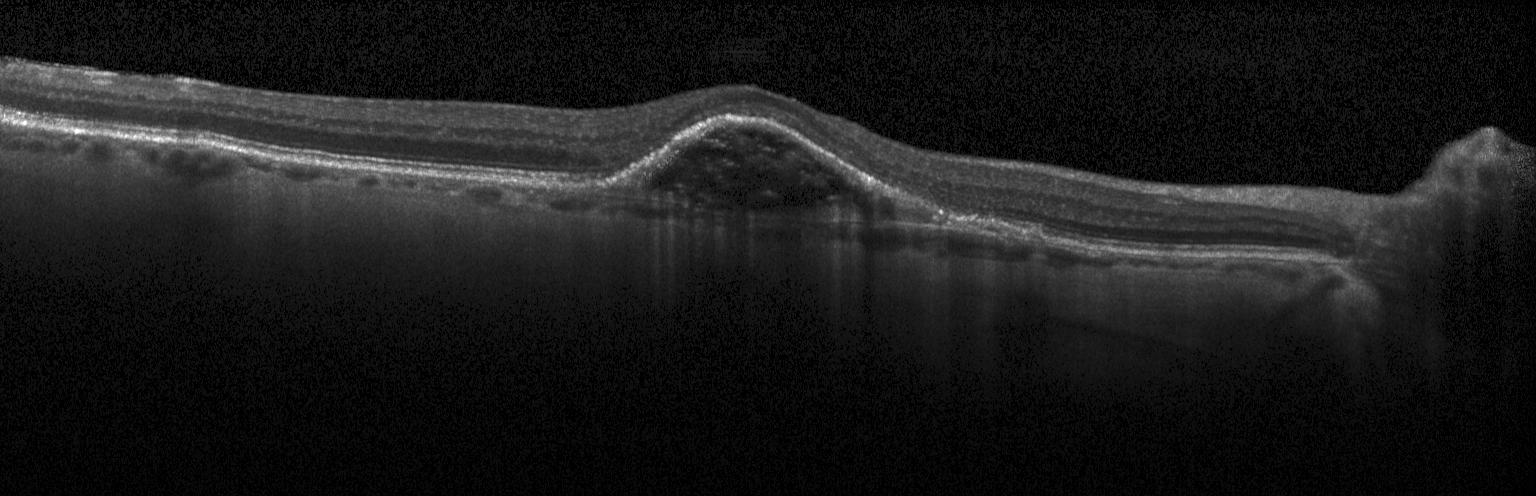

Horizontal scan through the fovea · optical coherence tomography scan · spectral-domain optical coherence tomography
Impression: a choroidal neovascular membrane.